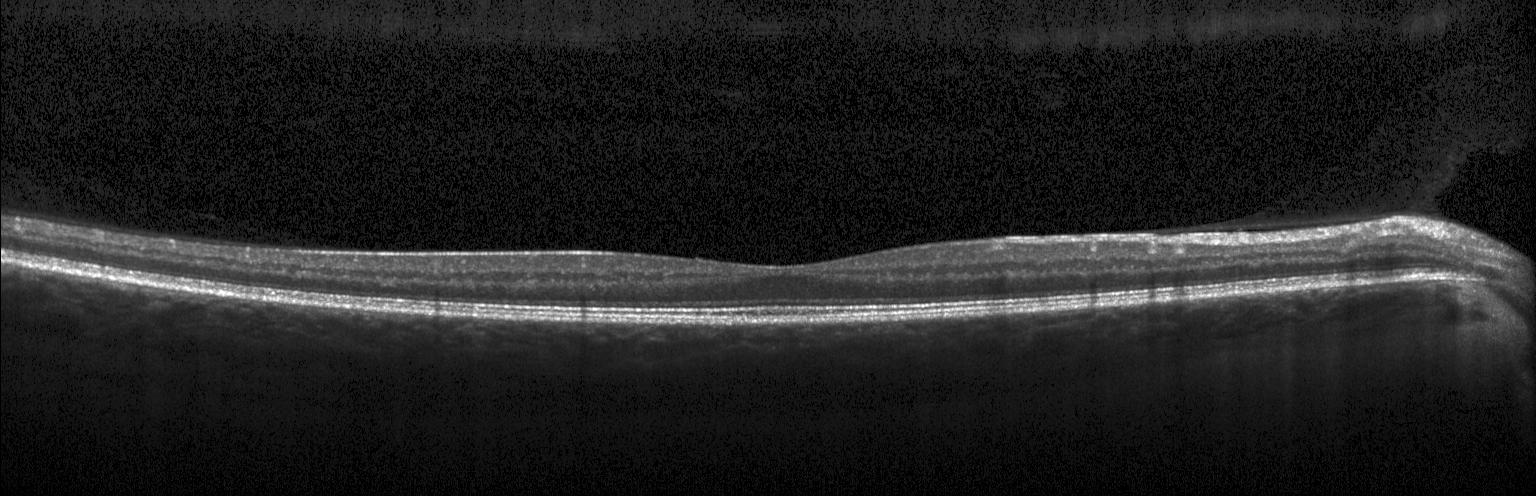

Finding: neither CNV, DME, nor drusen.